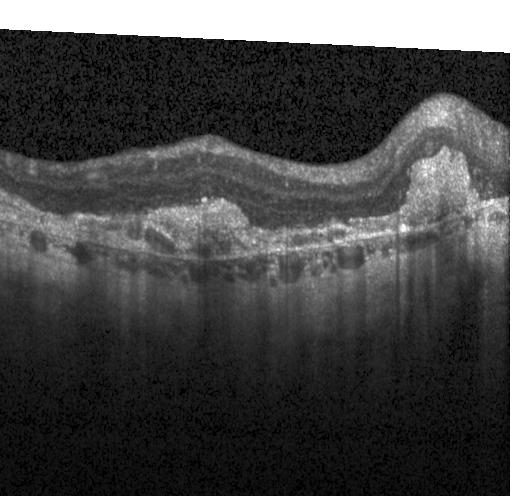 SD-OCT. Retinal OCT cross-section. Instrument: Heidelberg Spectralis
Assessment: choroidal neovascularization.